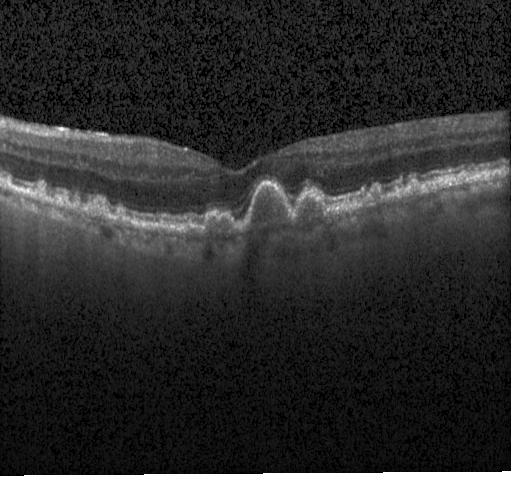 OCT line scan · through the macula · Heidelberg Spectralis OCT system.
Macular OCT: multiple drusen.